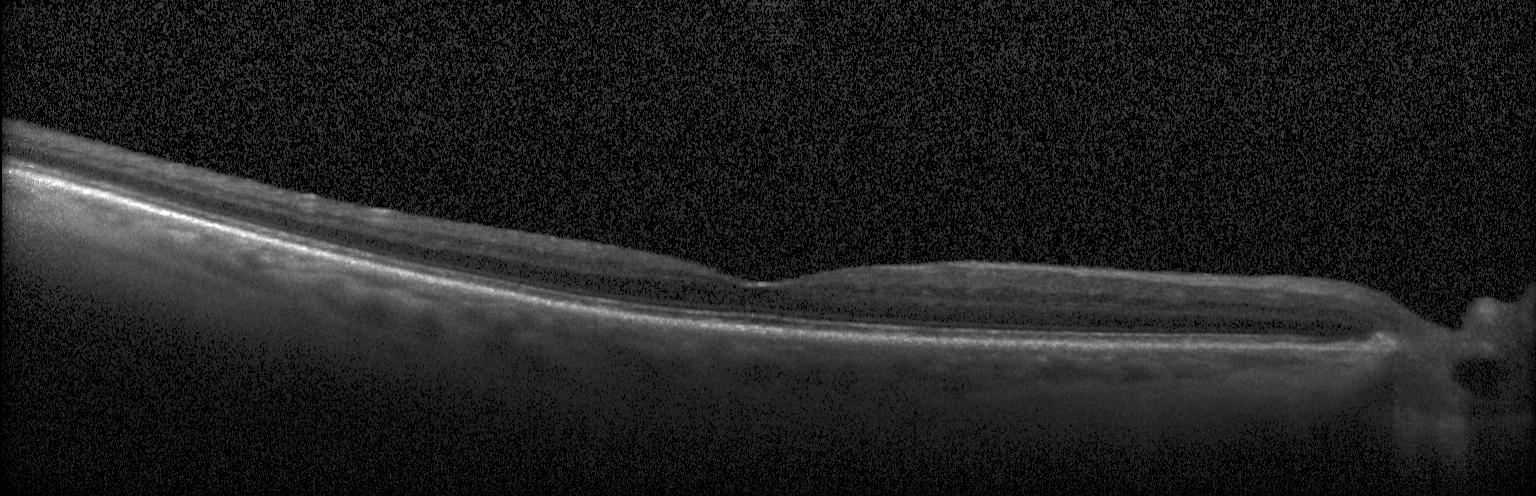
Diagnosis: no CNV, no DME, and no drusen.